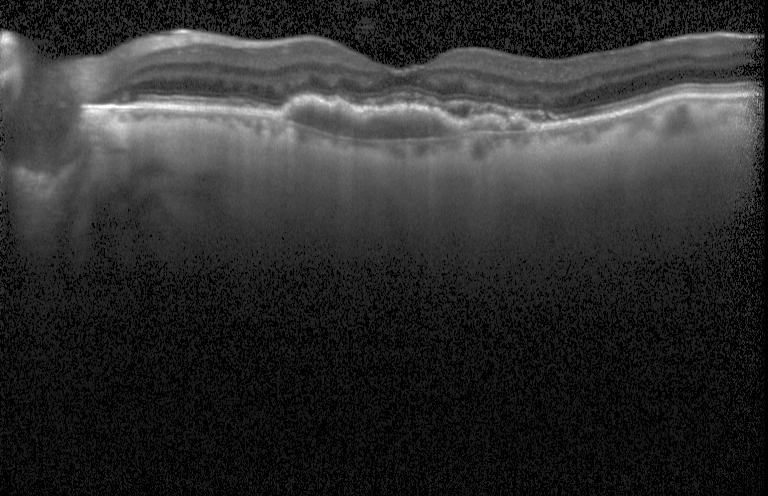 Macular OCT demonstrating a choroidal neovascular membrane.